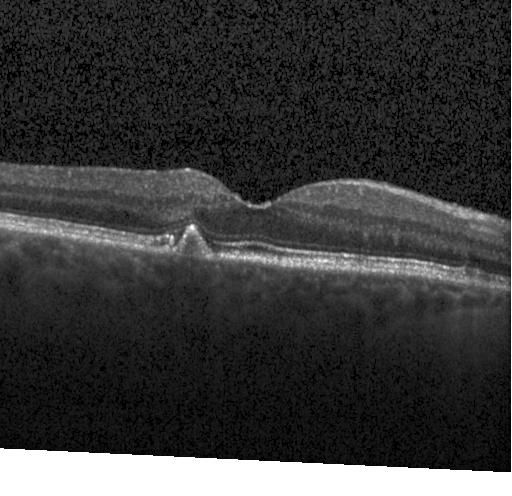

Heidelberg Spectralis, macular scan, retinal OCT B-scan, spectral-domain optical coherence tomography — Multiple drusen.